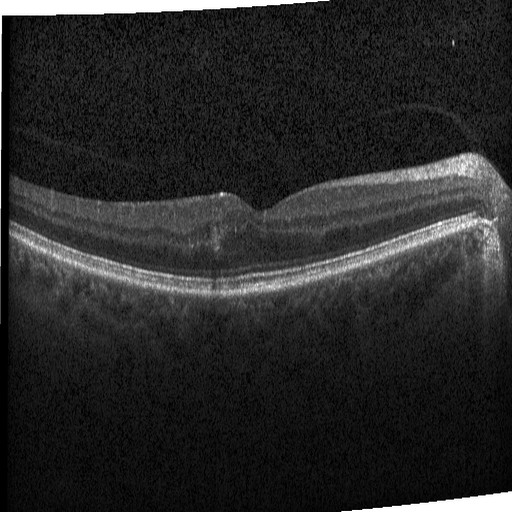

Spectral-domain OCT · instrument: Heidelberg Spectralis · optical coherence tomography scan — Diagnosis: diabetic macular edema (DME).